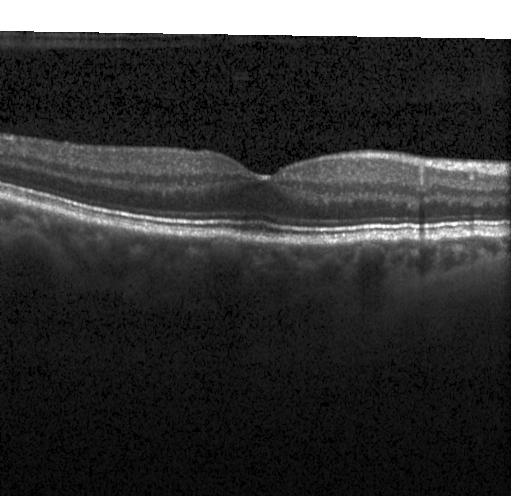

Impression: no evidence of choroidal neovascularization, diabetic macular edema, or drusen.